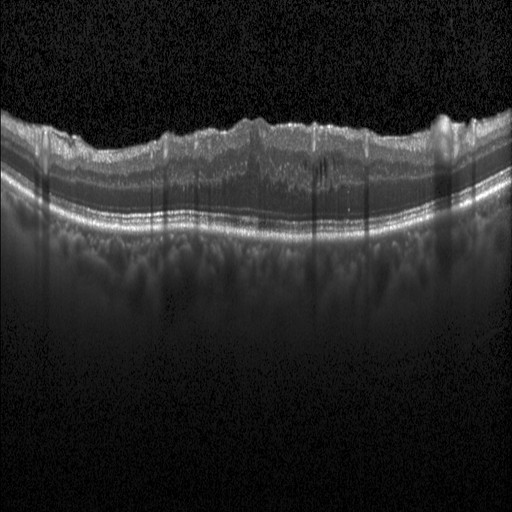

Diagnosis: diabetic macular edema (DME).